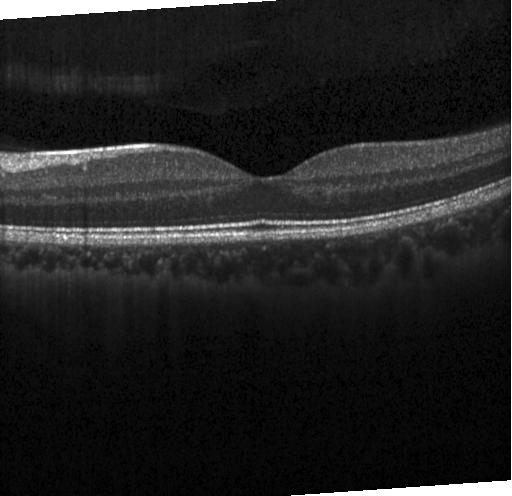 OCT line scan; horizontal scan through the fovea. Dx: neither CNV, DME, nor drusen.